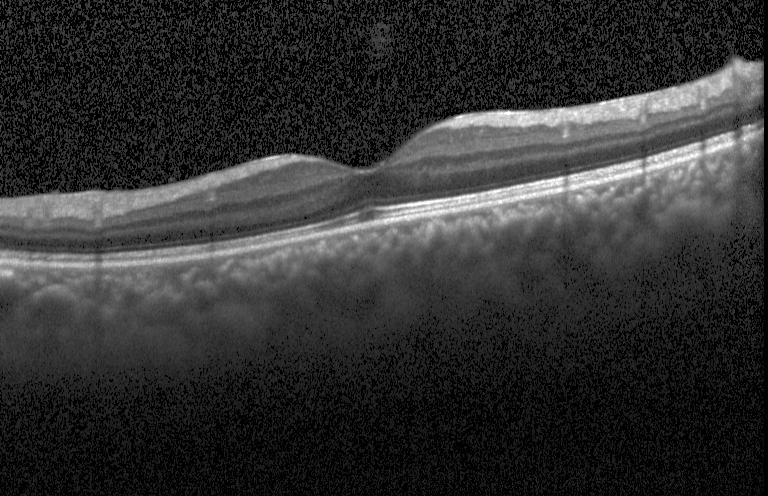 OCT scan showing no choroidal neovascularization, no diabetic macular edema, and no drusen.